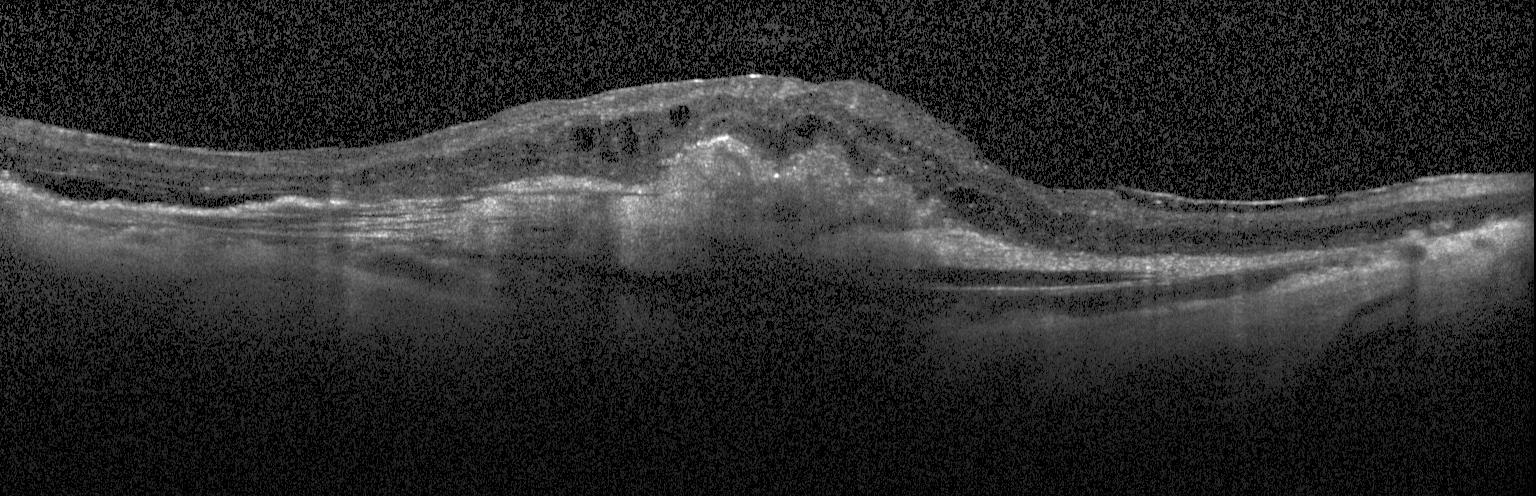 Instrument: Heidelberg Spectralis; optical coherence tomography scan.
Dx: a choroidal neovascular membrane.